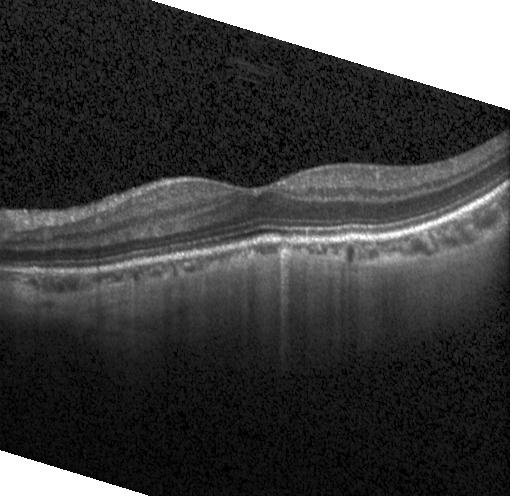

Fovea-centered, Heidelberg Spectralis OCT system, retinal OCT B-scan
This B-scan demonstrates no choroidal neovascularization, no diabetic macular edema, and no drusen.